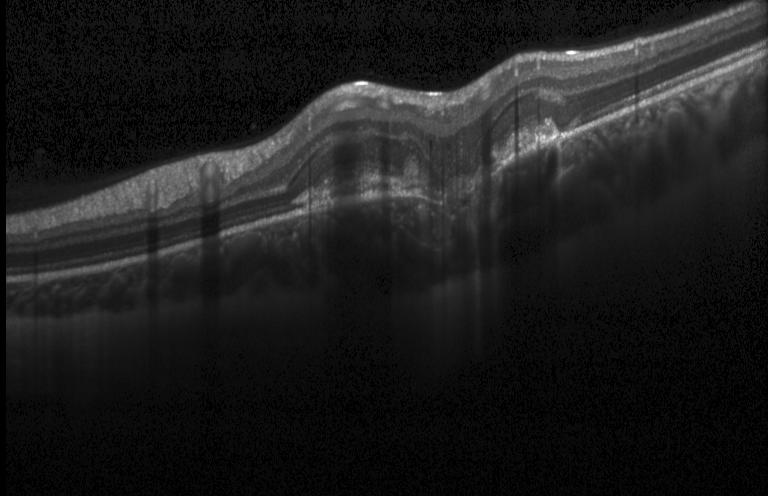
Optical coherence tomography scan; centered on the fovea. Finding: a choroidal neovascular membrane.